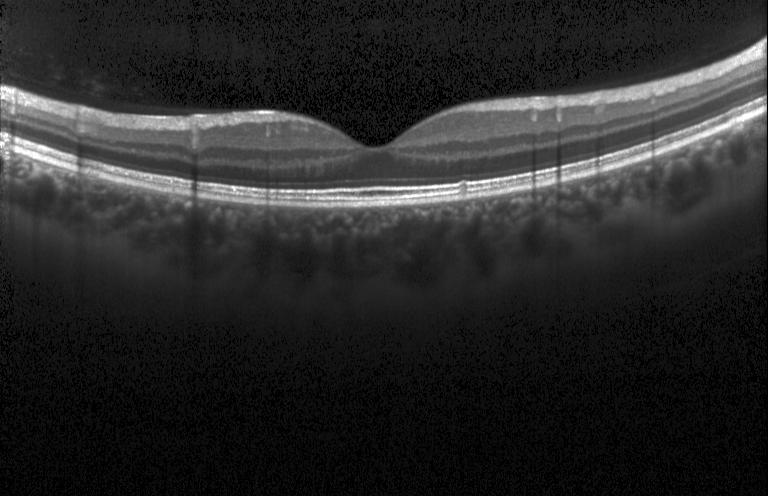

Finding: neither choroidal neovascularization, diabetic macular edema, nor drusen.